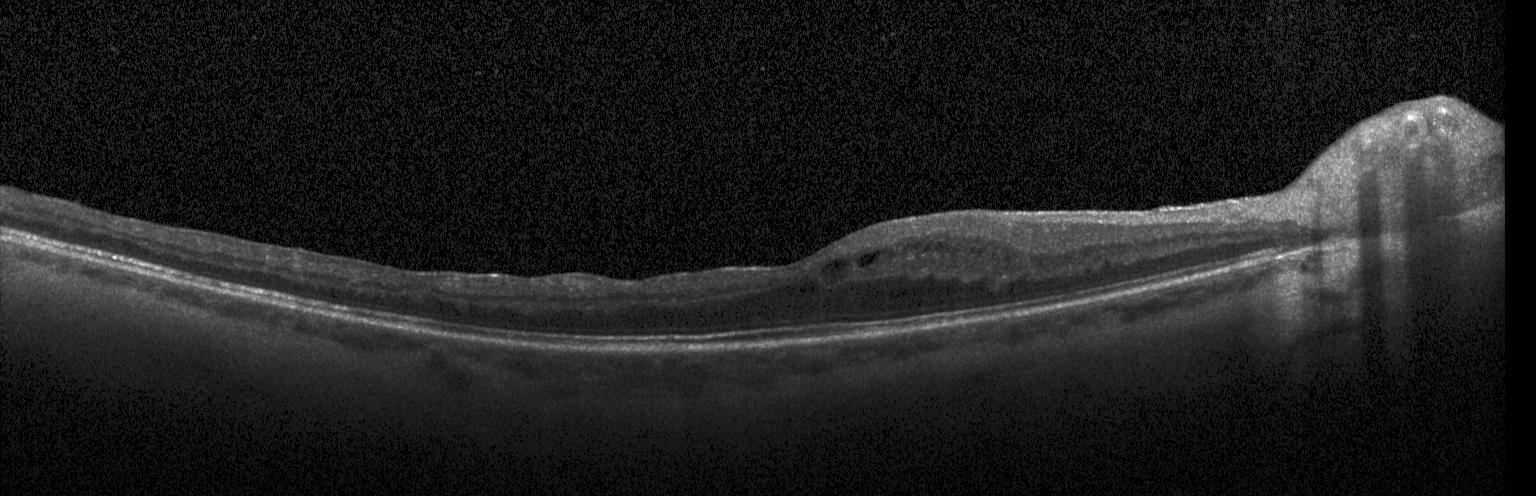

Retinal OCT cross-section showing diabetic macular edema.